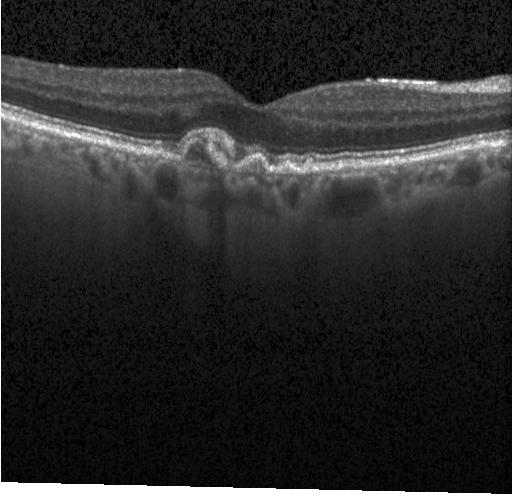

Optical coherence tomography B-scan. Choroidal neovascularization.